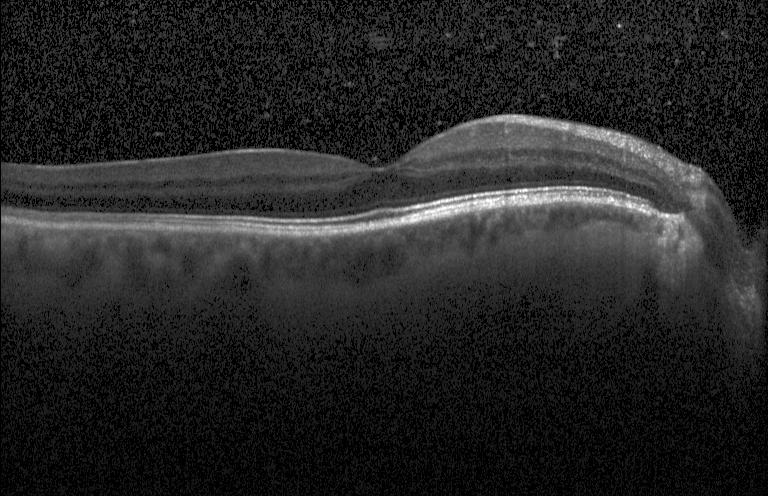

OCT line scan; SD-OCT; Heidelberg Spectralis; horizontal scan through the fovea.
Finding: no evidence of CNV, DME, or drusen.